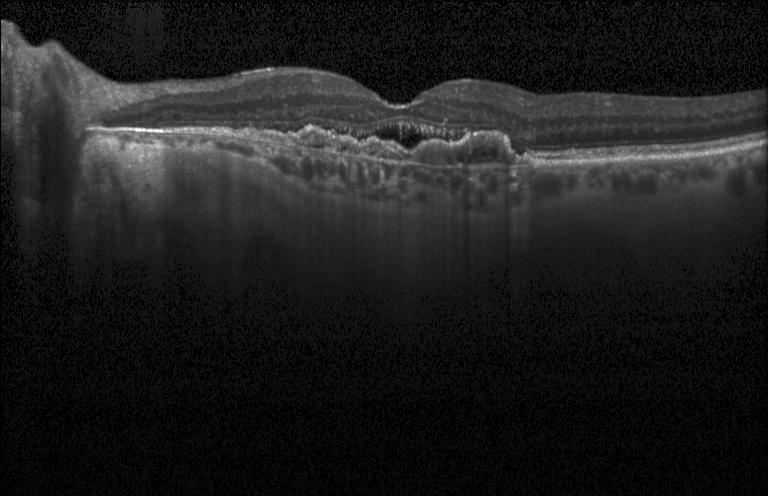

OCT line scan · spectral-domain optical coherence tomography — Impression: a choroidal neovascular membrane.